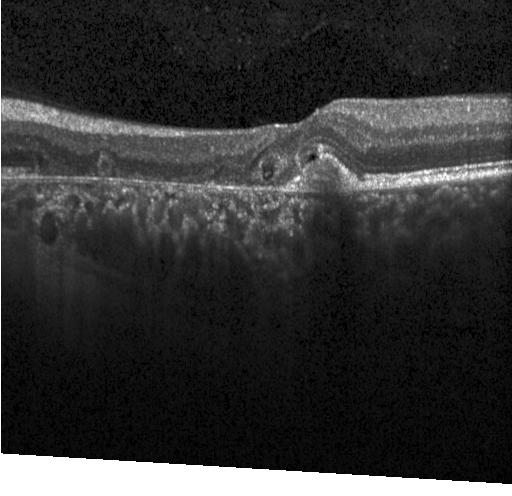 Acquired on a Heidelberg Spectralis; retinal OCT B-scan; spectral-domain OCT — This B-scan demonstrates a choroidal neovascular membrane.